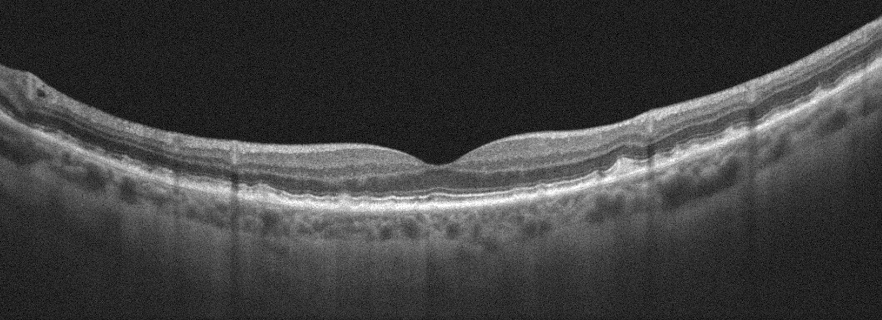 Oculus dexter; macular scan; instrument: Optovue Avanti RTVue XR; OCT B-scan
Age-related macular degeneration (AMD).